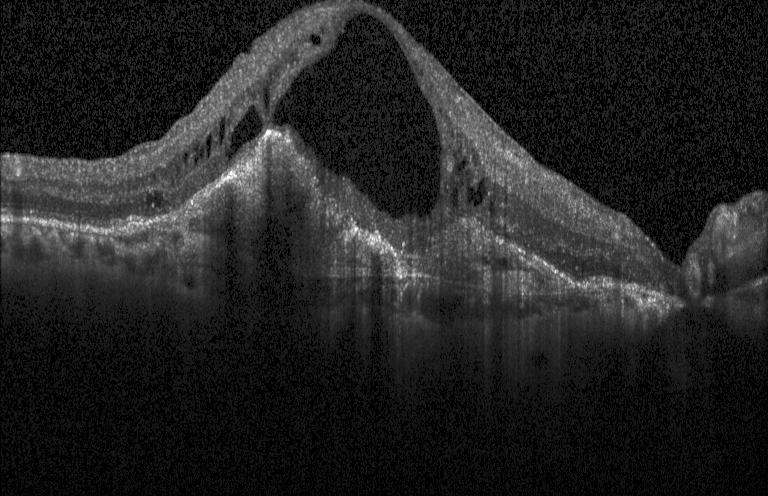
Retinal OCT B-scan. SD-OCT
Finding: a choroidal neovascular membrane.